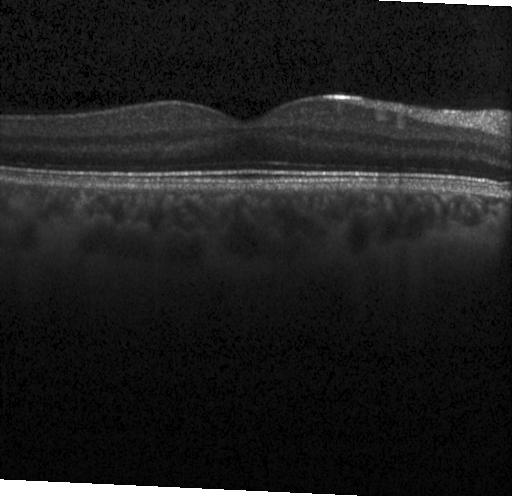
Instrument: Heidelberg Spectralis, spectral-domain OCT, through the macula, OCT line scan. No choroidal neovascularization, diabetic macular edema, or drusen.